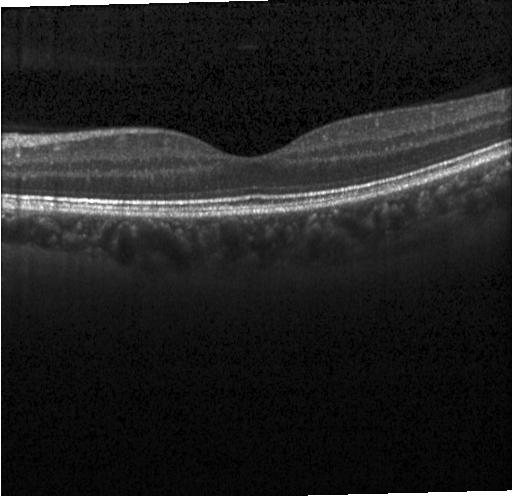

Macular OCT demonstrating neither CNV, DME, nor drusen.